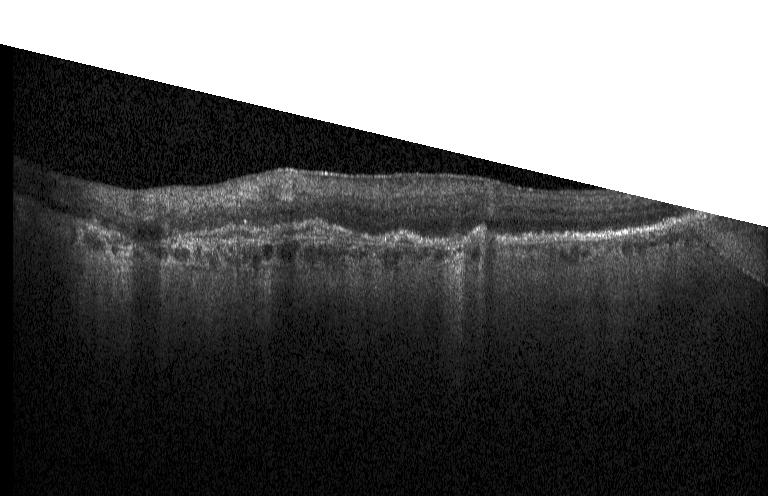 Retinal OCT cross-section showing choroidal neovascularization (CNV).